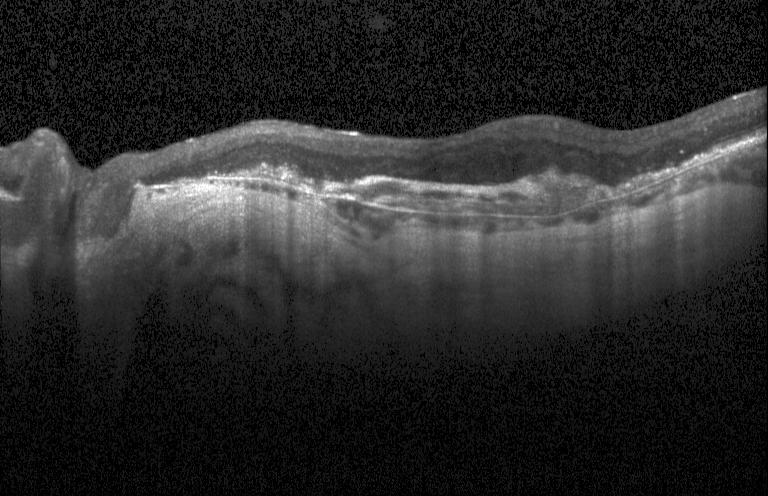

SD-OCT. Optical coherence tomography scan
Assessment: a choroidal neovascular membrane.